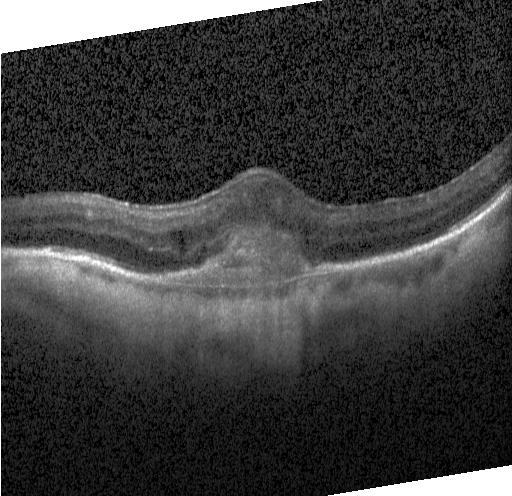
OCT line scan · instrument: Heidelberg Spectralis · centered on the fovea.
Finding: choroidal neovascularization (CNV).